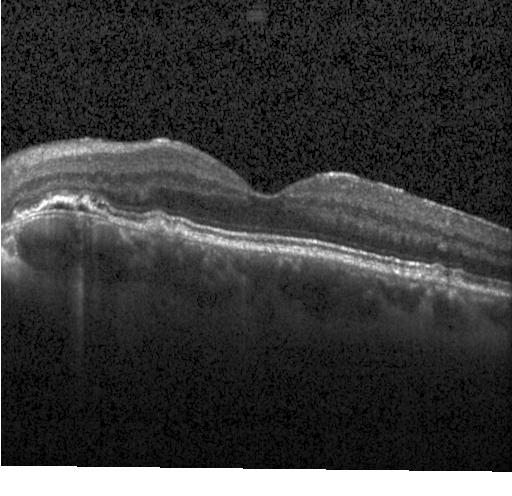 Retinal OCT B-scan; fovea-centered; acquired on a Heidelberg Spectralis — This B-scan demonstrates sub-RPE drusenoid deposits.